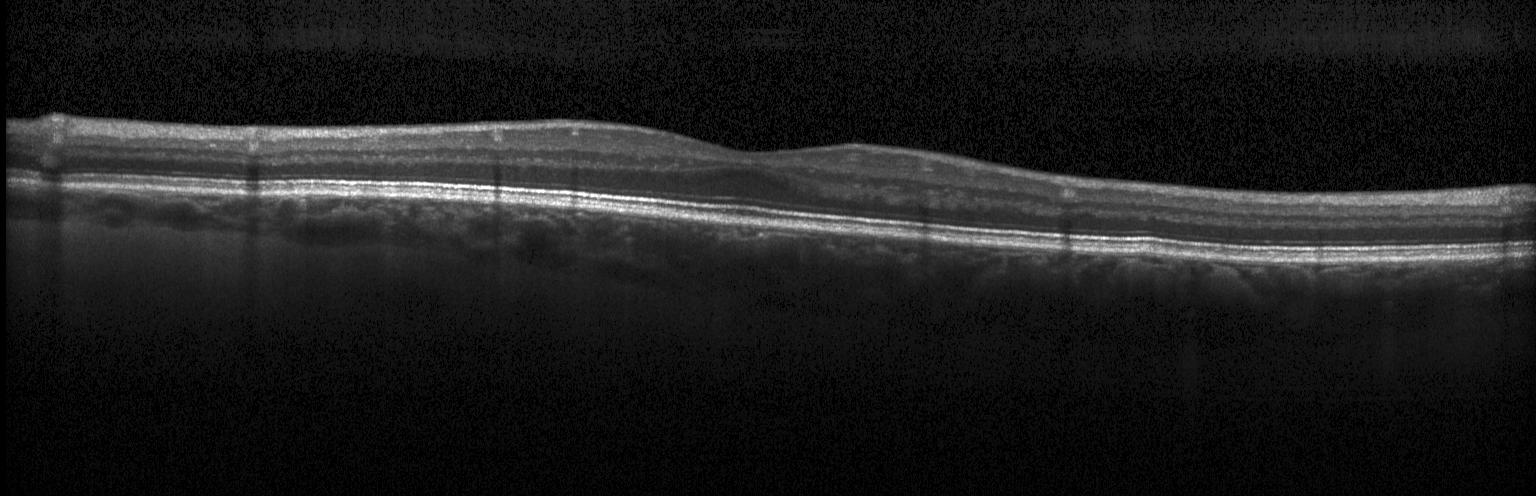 OCT B-scan · spectral-domain optical coherence tomography
Assessment: no evidence of CNV, DME, or drusen.